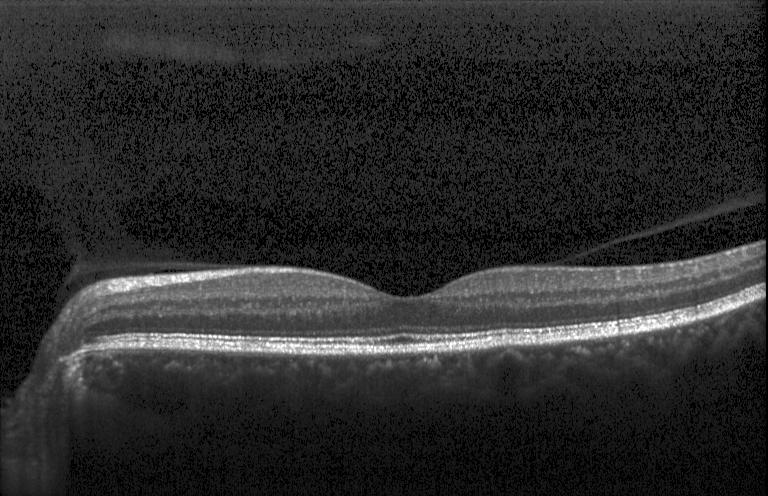
Assessment: no evidence of CNV, DME, or drusen.